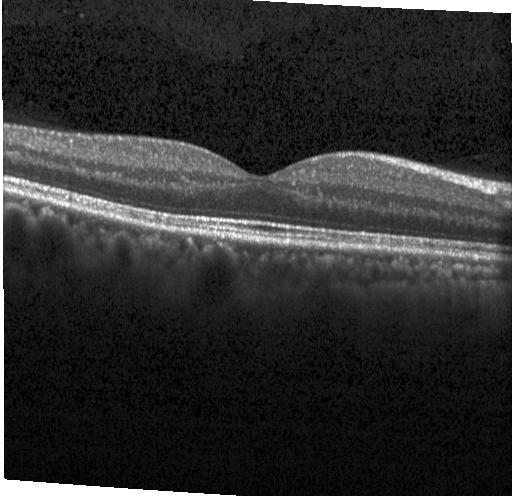

The scan shows no evidence of choroidal neovascularization, diabetic macular edema, or drusen.